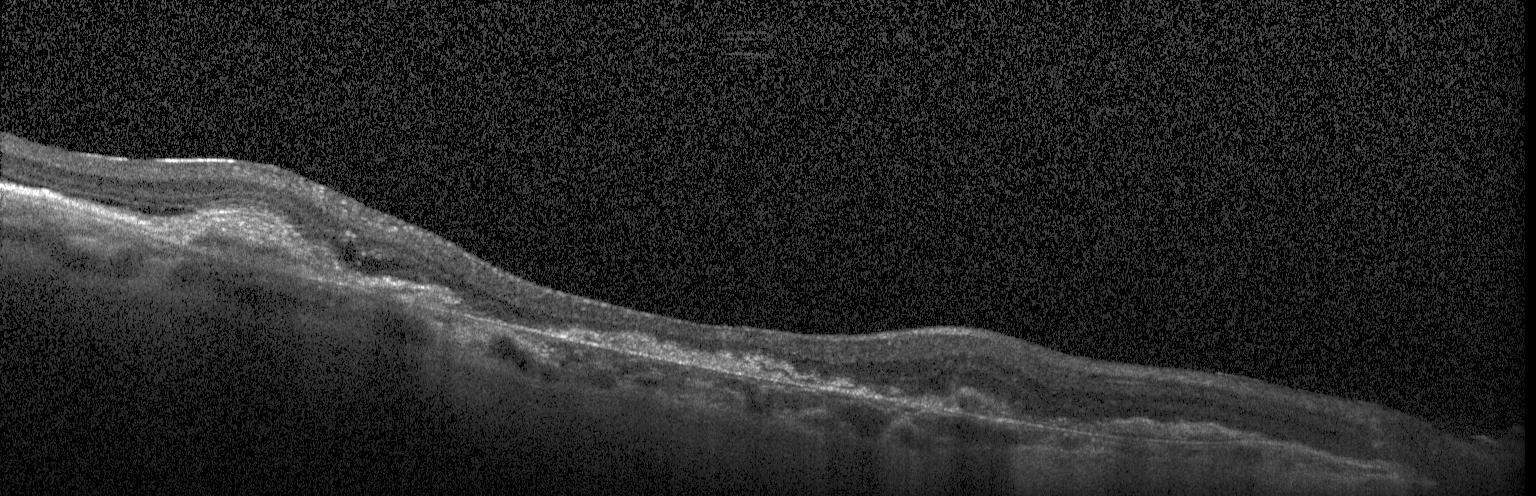 Acquired on a Heidelberg Spectralis; SD-OCT; optical coherence tomography B-scan — OCT finding: choroidal neovascularization.